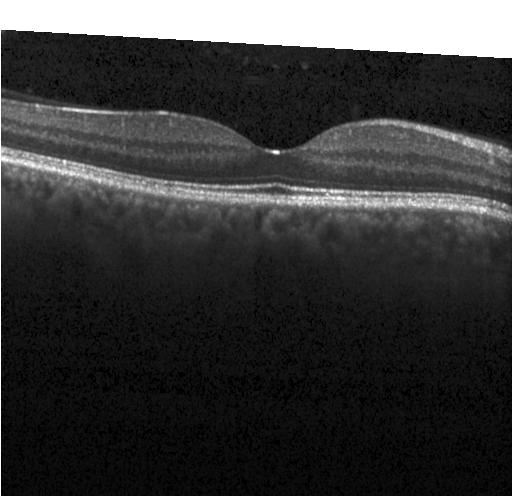 OCT line scan, SD-OCT, acquired on a Heidelberg Spectralis, centered on the fovea
Diagnosis: no choroidal neovascularization, diabetic macular edema, or drusen.